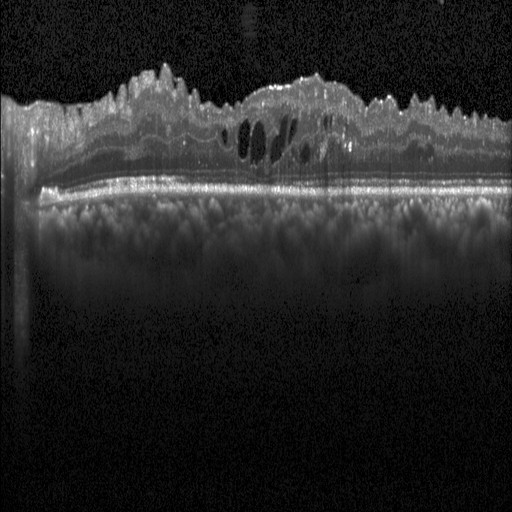 Optical coherence tomography scan, horizontal scan through the fovea
Dx: DME.